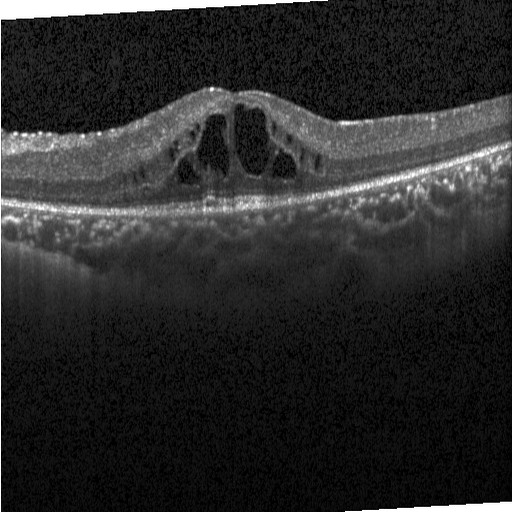
Heidelberg Spectralis OCT system; retinal OCT B-scan; centered on the fovea; SD-OCT
Finding: diabetic macular edema.